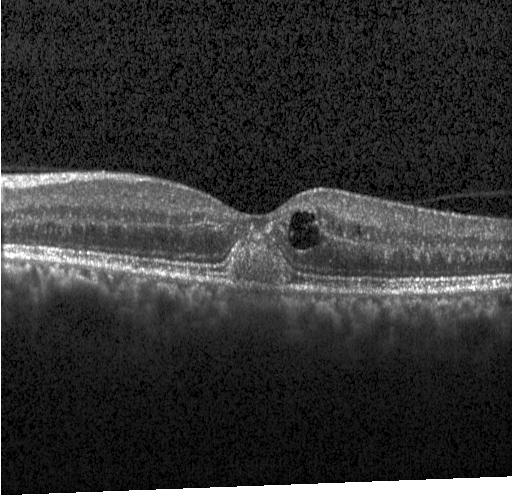

Optical coherence tomography B-scan, Heidelberg Spectralis OCT system — Diagnosis: CNV.